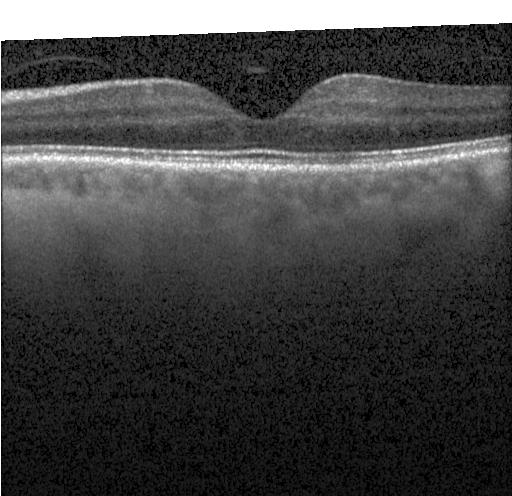 Spectral-domain OCT · optical coherence tomography B-scan · Heidelberg Spectralis · through the macula.
Dx: no choroidal neovascularization, no diabetic macular edema, and no drusen.